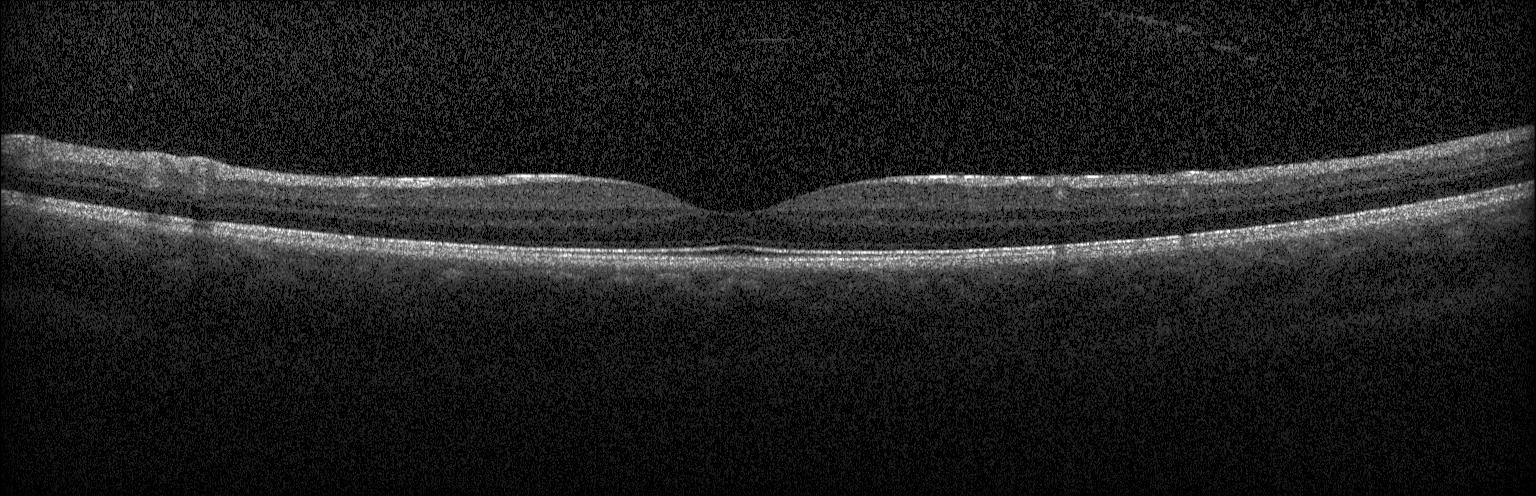

Macular OCT: neither CNV, DME, nor drusen.